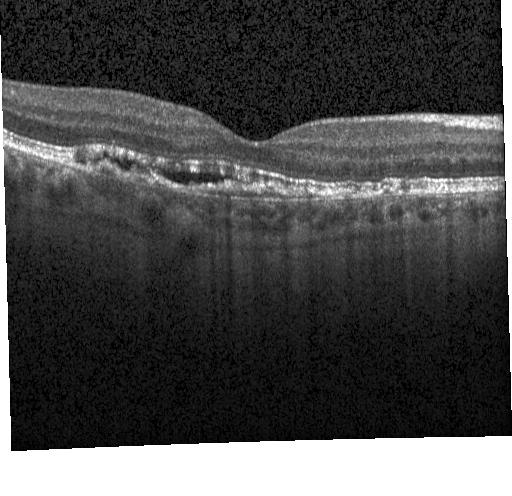

Heidelberg Spectralis OCT system, centered on the fovea, spectral-domain OCT, OCT line scan.
Impression: choroidal neovascularization.